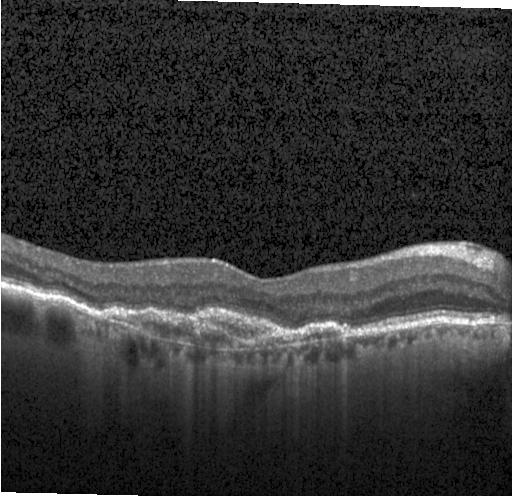

Heidelberg Spectralis OCT system · centered on the fovea · spectral-domain OCT · retinal OCT cross-section
Impression: choroidal neovascularization (CNV).